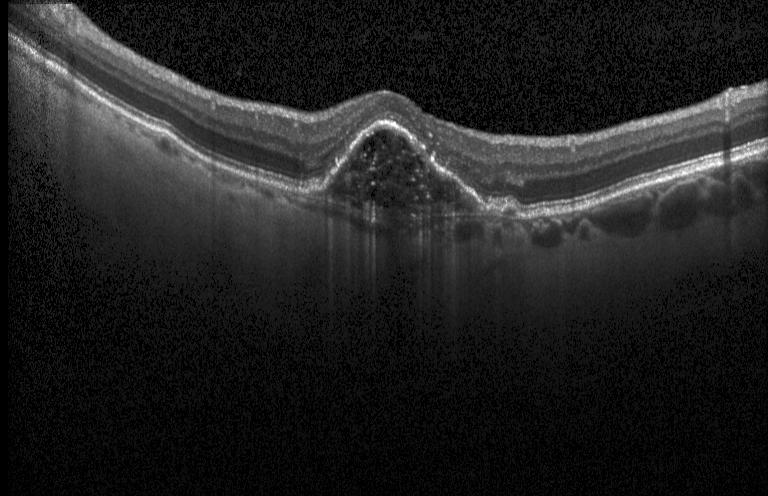

Finding: choroidal neovascularization.